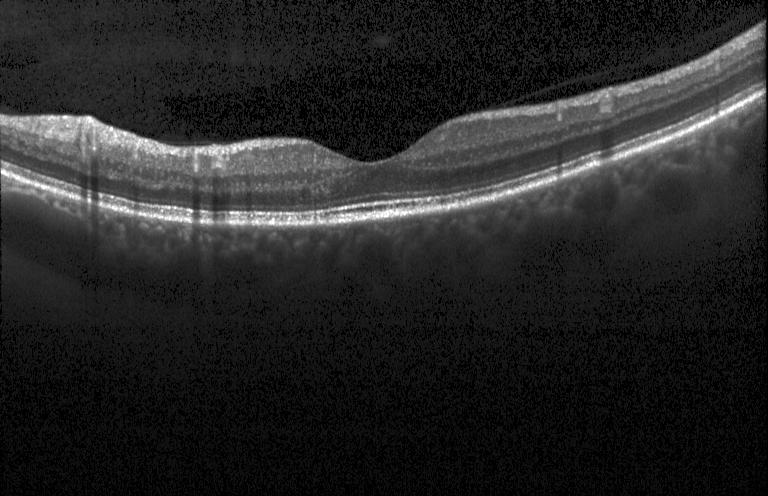
Optical coherence tomography scan.
Dx: neither choroidal neovascularization, diabetic macular edema, nor drusen.